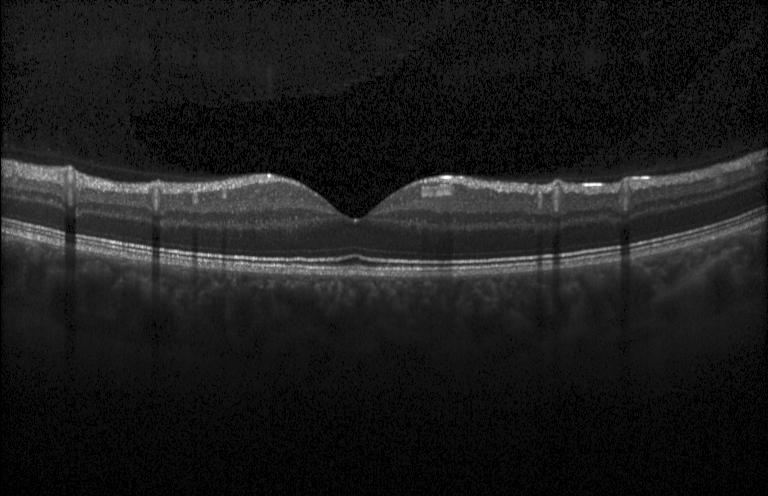 Finding: no choroidal neovascularization, diabetic macular edema, or drusen.